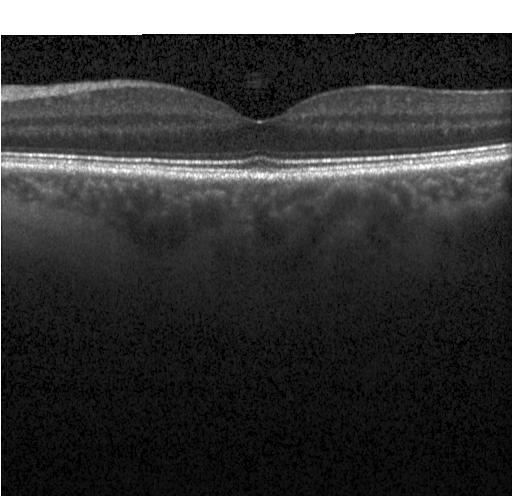
SD-OCT, macular scan, instrument: Heidelberg Spectralis, OCT B-scan.
Assessment: no evidence of choroidal neovascularization, diabetic macular edema, or drusen.